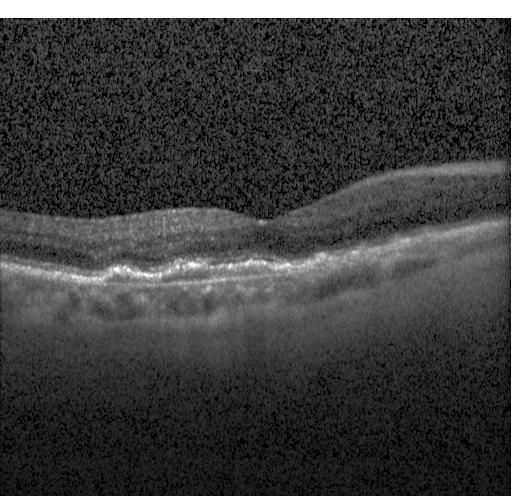
Finding: choroidal neovascularization (CNV).